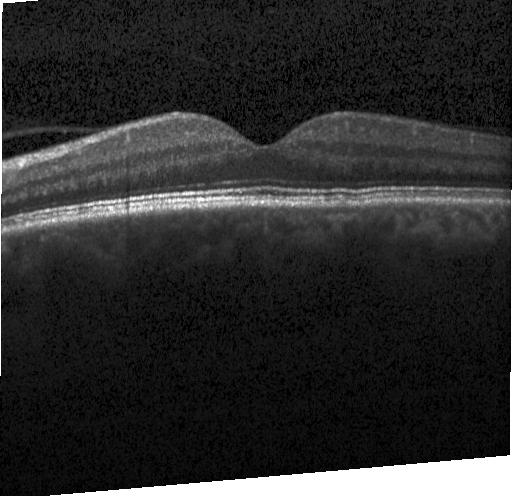
Impression: no choroidal neovascularization, diabetic macular edema, or drusen.